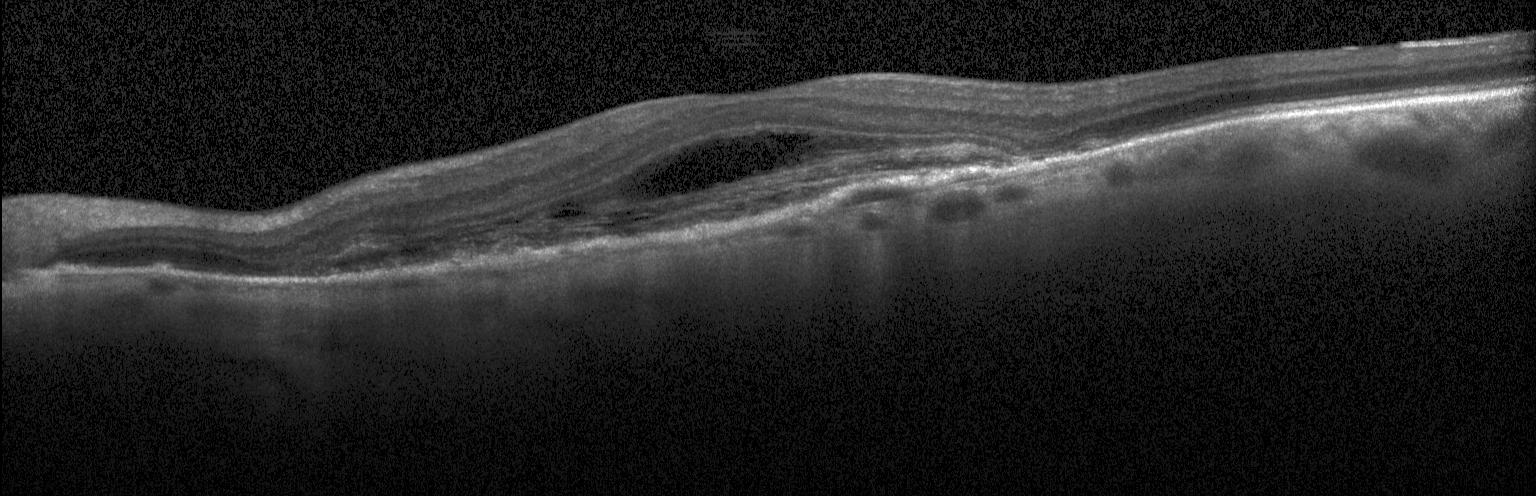 Retinal OCT cross-section.
Finding: a choroidal neovascular membrane.